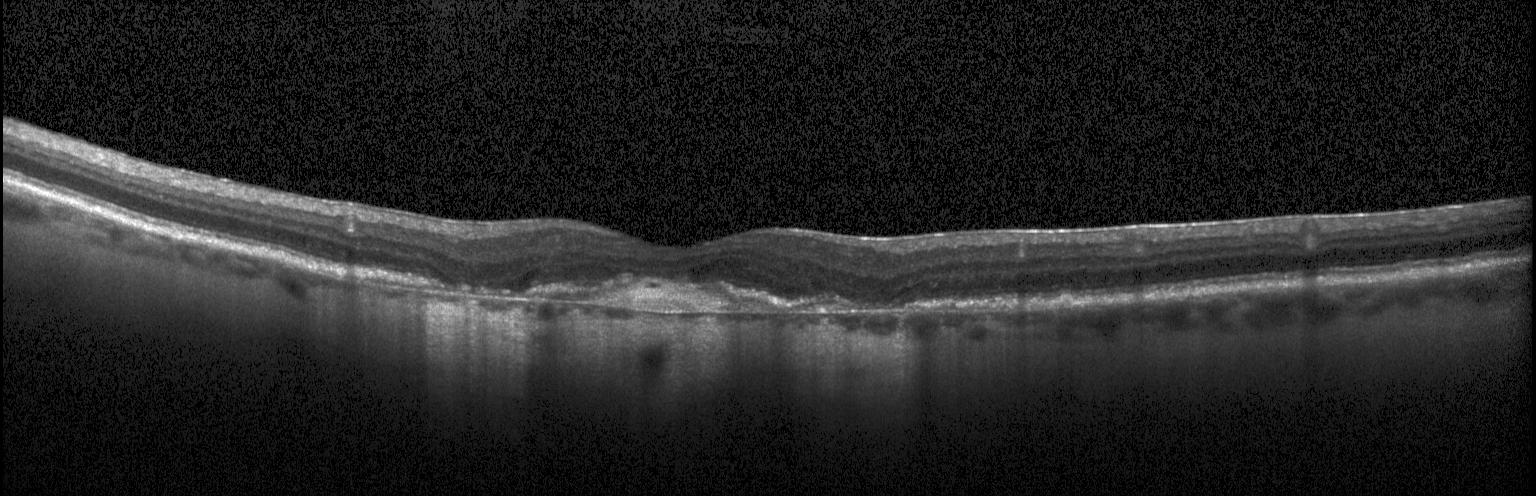 Diagnosis: a choroidal neovascular membrane.